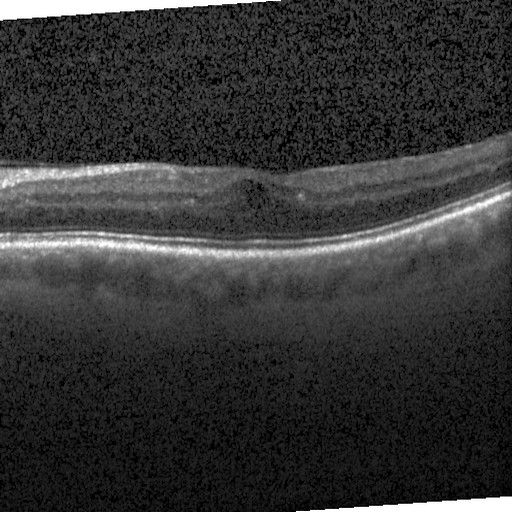
Heidelberg Spectralis OCT system, through the macula, spectral-domain optical coherence tomography, retinal OCT cross-section — Dx: diabetic macular edema.